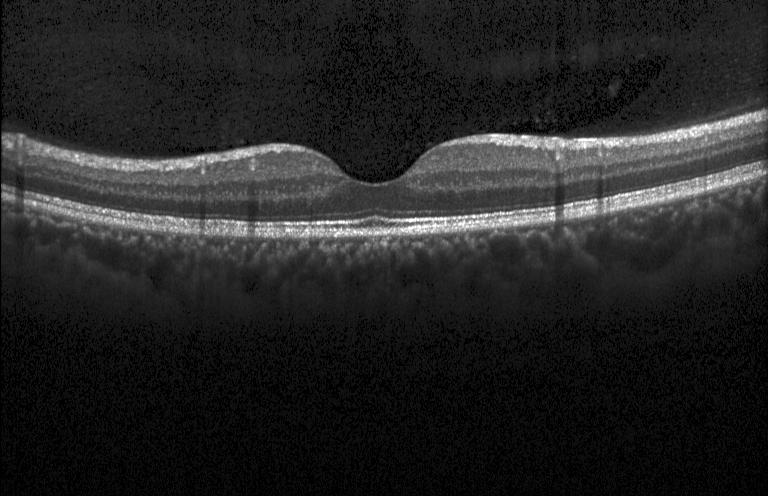 This B-scan demonstrates neither CNV, DME, nor drusen.